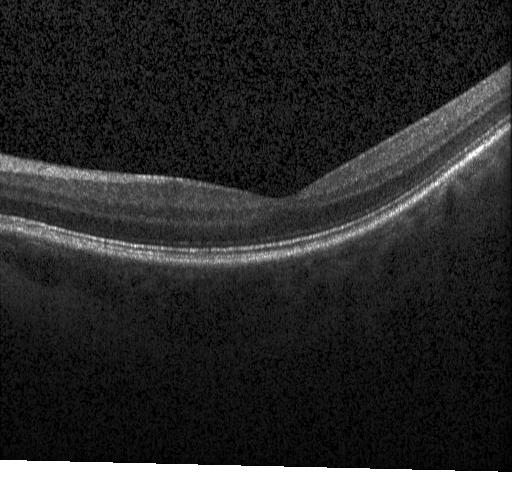 Macular OCT demonstrating no CNV, no DME, and no drusen.